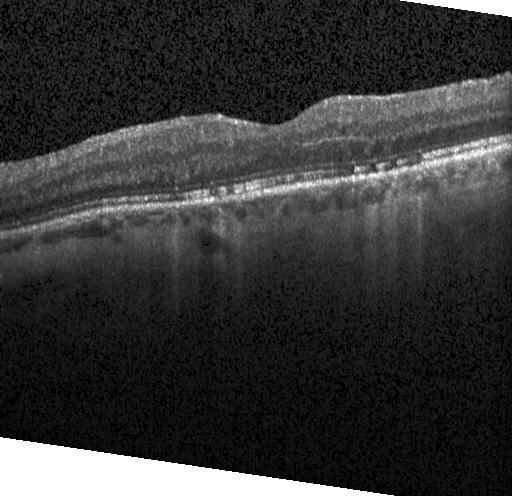

Horizontal scan through the fovea. Optical coherence tomography B-scan. SD-OCT. Instrument: Heidelberg Spectralis — No choroidal neovascularization, diabetic macular edema, or drusen.